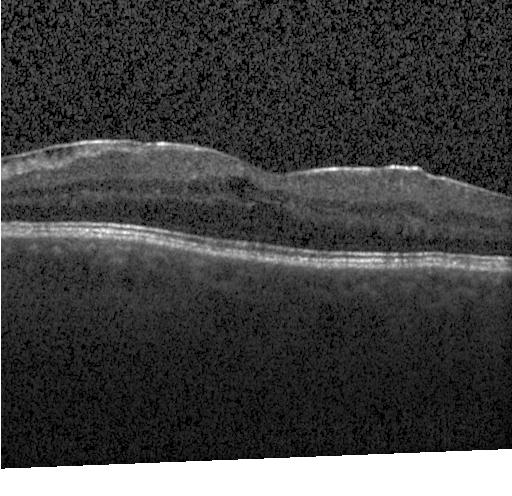 Diabetic macular edema (DME).